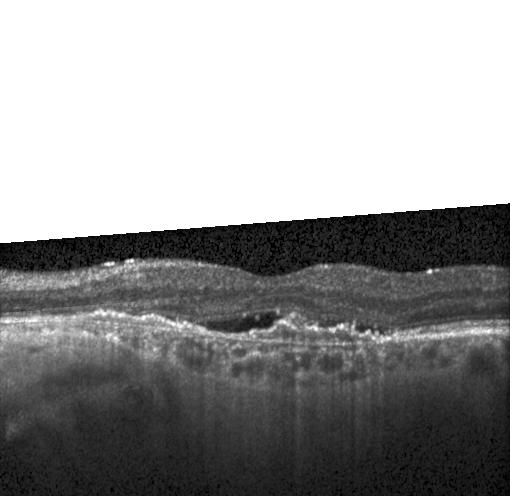 Choroidal neovascularization.